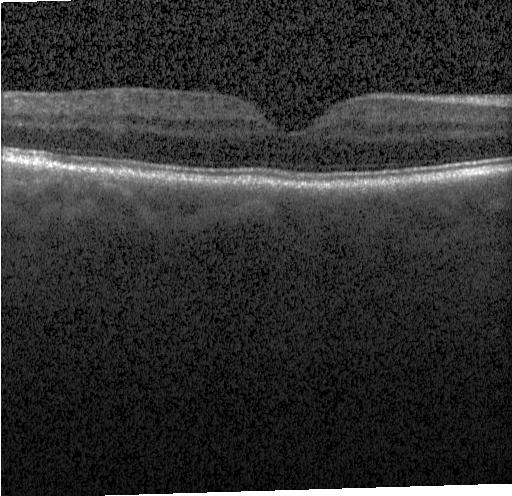

Diagnosis: no evidence of choroidal neovascularization, diabetic macular edema, or drusen.